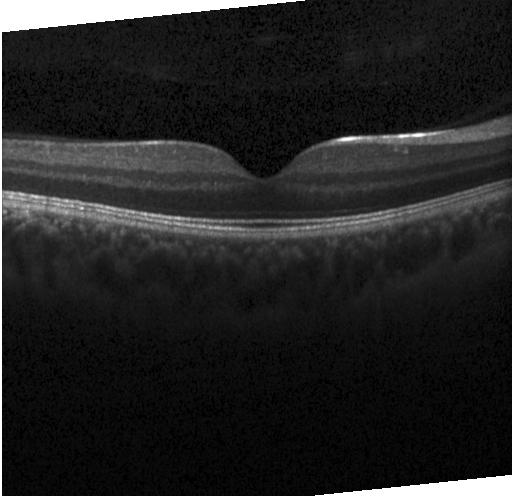 Finding: no evidence of CNV, DME, or drusen.